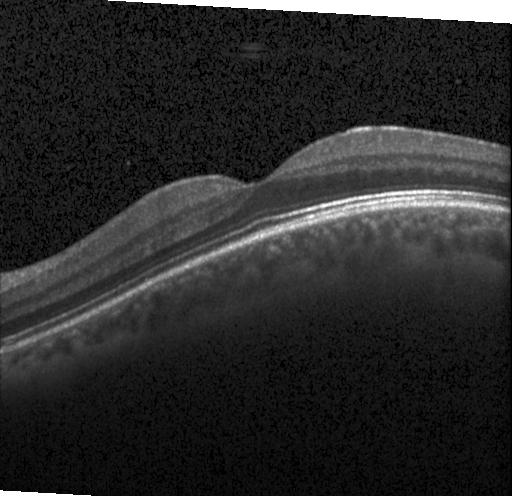 Instrument: Heidelberg Spectralis. Optical coherence tomography B-scan. Spectral-domain OCT. This B-scan demonstrates no evidence of CNV, DME, or drusen.